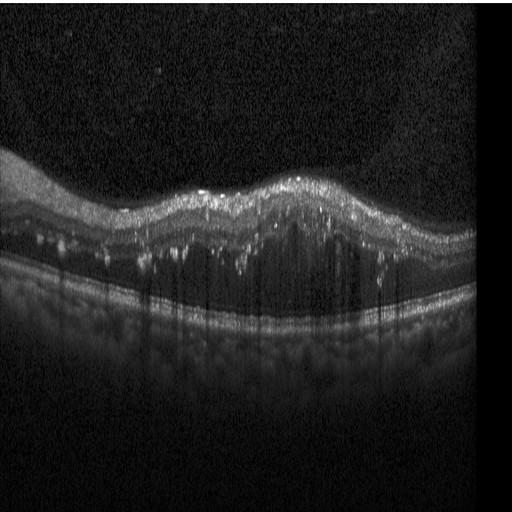 OCT B-scan; SD-OCT; fovea-centered — Diagnosis: DME.